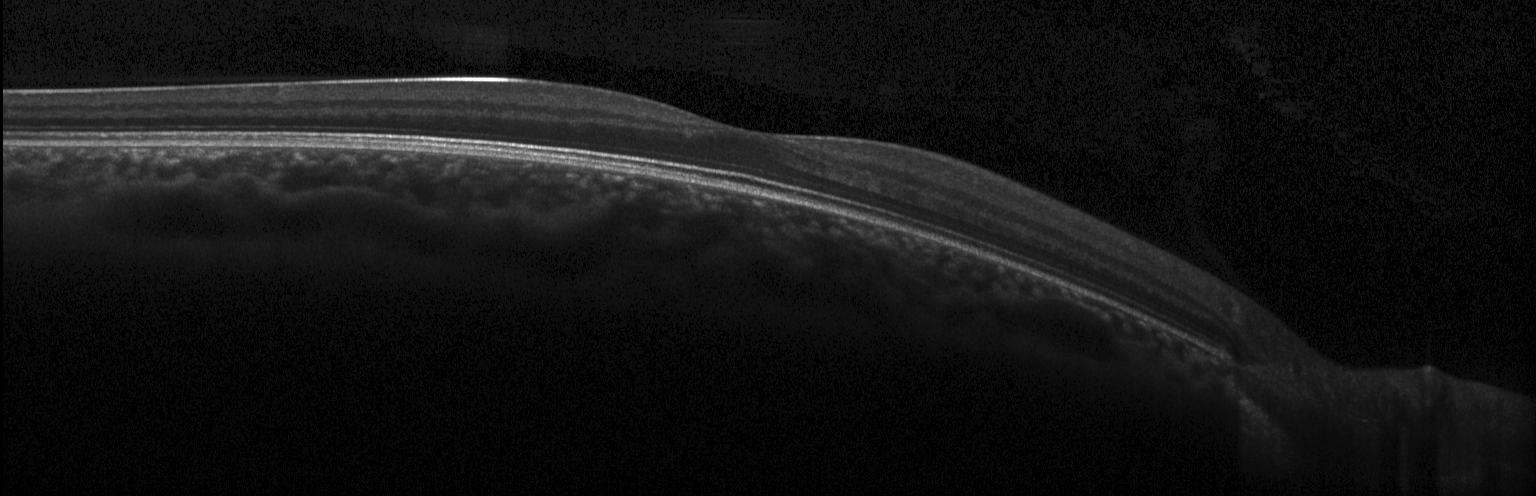
Heidelberg Spectralis OCT system, optical coherence tomography scan, spectral-domain OCT. This B-scan demonstrates no evidence of CNV, DME, or drusen.